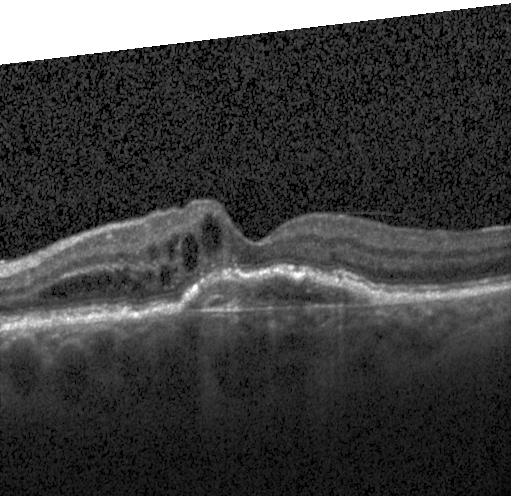 Acquired on a Heidelberg Spectralis, retinal OCT cross-section — Finding: CNV.